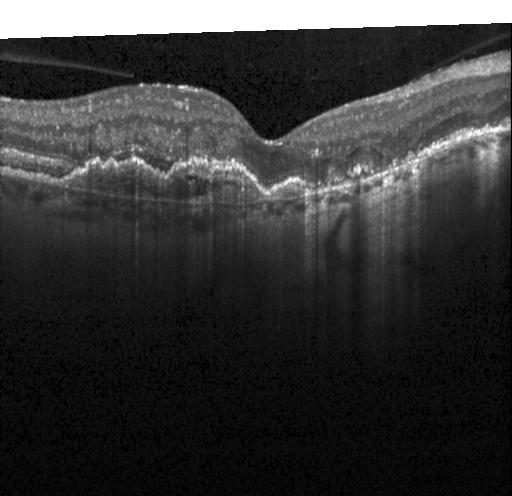
Retinal OCT cross-section showing a choroidal neovascular membrane.